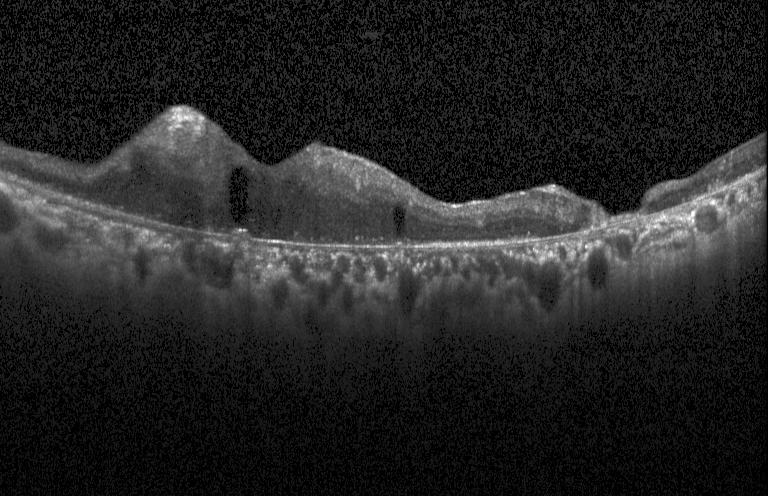
Optical coherence tomography B-scan; through the macula; spectral-domain OCT; acquired on a Heidelberg Spectralis. This B-scan demonstrates a choroidal neovascular membrane.